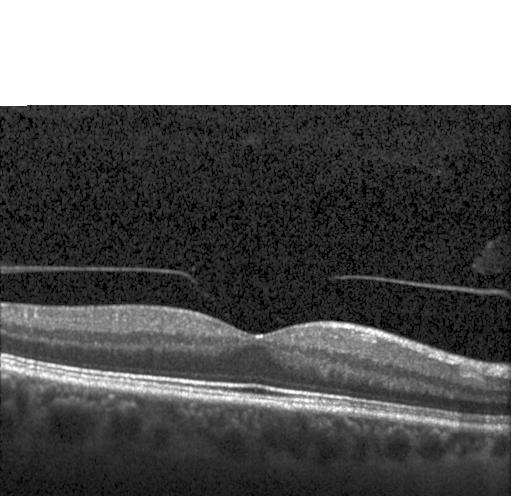 The scan shows no evidence of choroidal neovascularization, diabetic macular edema, or drusen.